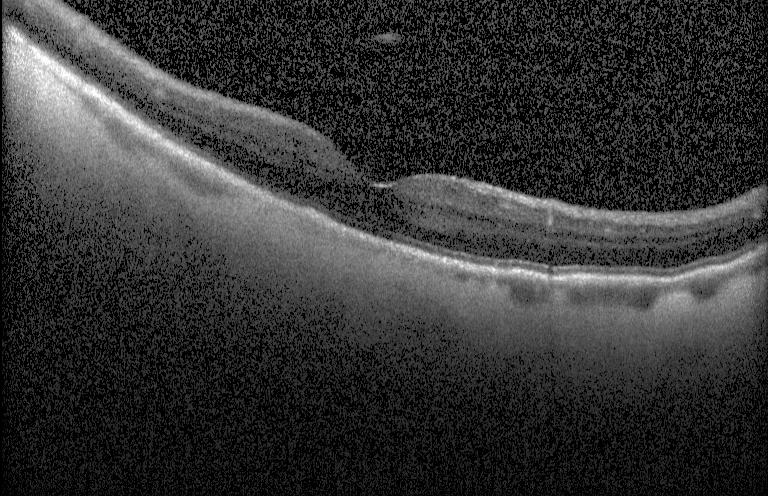
Spectral-domain OCT; horizontal scan through the fovea; retinal OCT B-scan. OCT finding: DME.